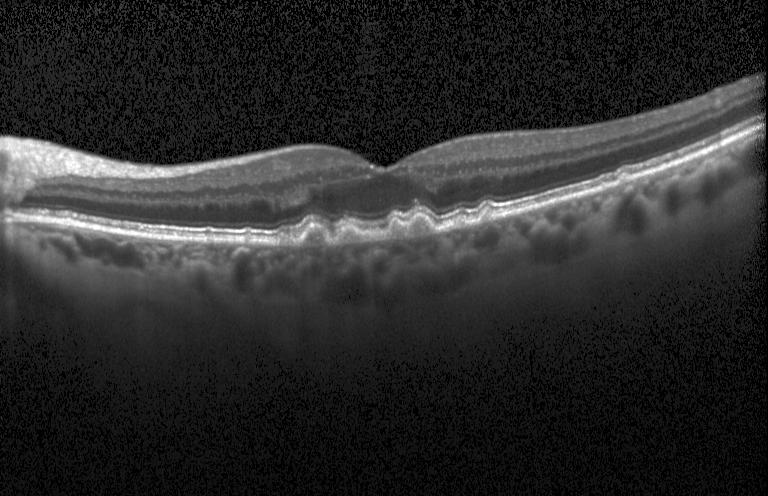 Horizontal scan through the fovea. Spectral-domain OCT. OCT line scan. Heidelberg Spectralis. Diagnosis: sub-RPE drusenoid deposits.